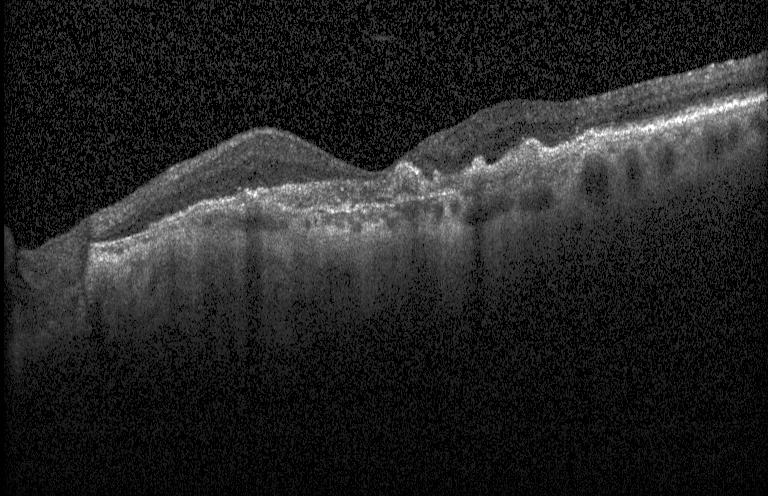

SD-OCT. Optical coherence tomography scan. Macular scan. Instrument: Heidelberg Spectralis — Dx: CNV.